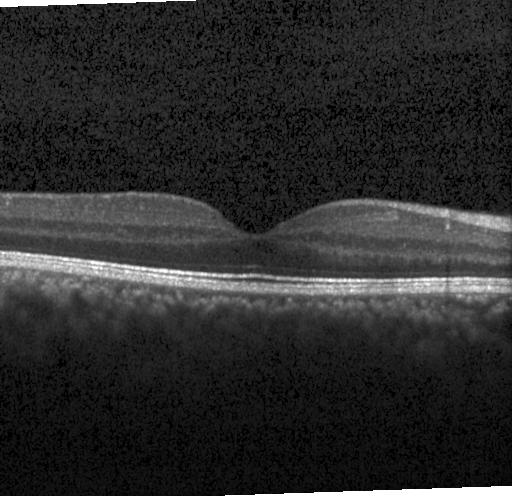 Retinal OCT cross-section. The scan shows no evidence of choroidal neovascularization, diabetic macular edema, or drusen.